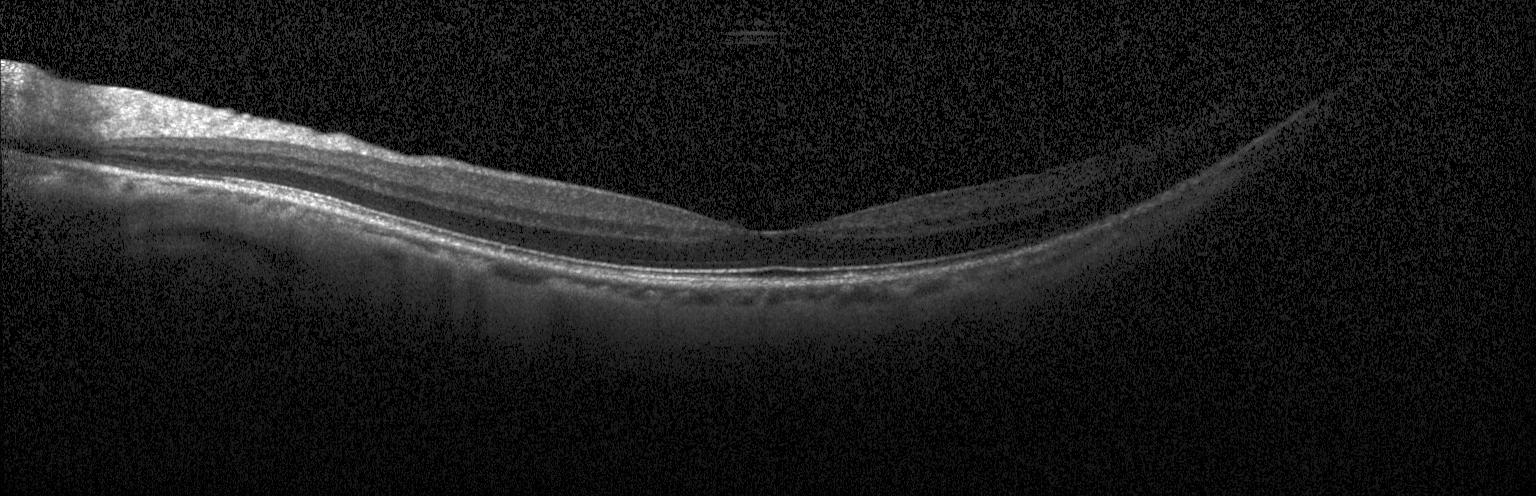 Macular OCT: neither choroidal neovascularization, diabetic macular edema, nor drusen.